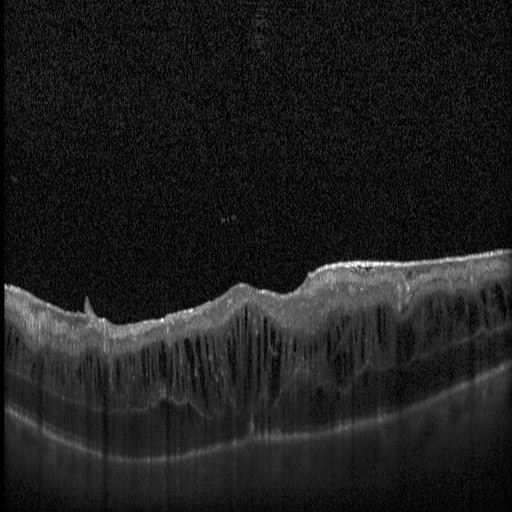 Macular scan, OCT B-scan, Heidelberg Spectralis OCT system, spectral-domain optical coherence tomography.
Assessment: diabetic macular edema.